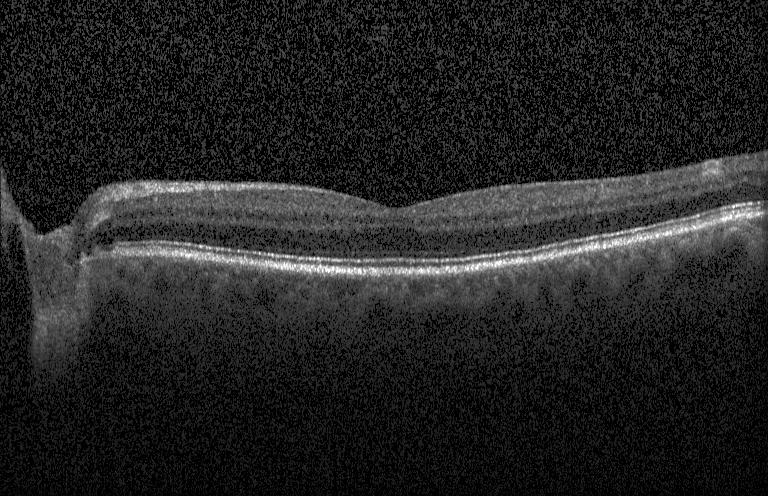
Assessment: no evidence of CNV, DME, or drusen.